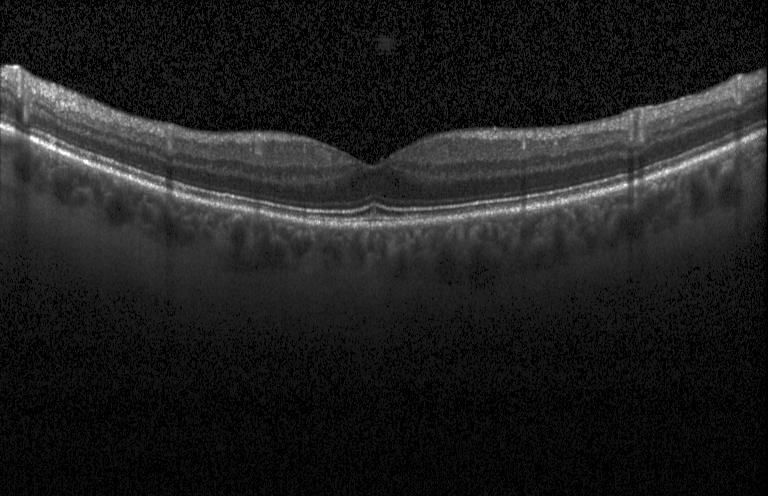

Retinal OCT cross-section · Heidelberg Spectralis OCT system · spectral-domain OCT
OCT finding: no CNV, no DME, and no drusen.